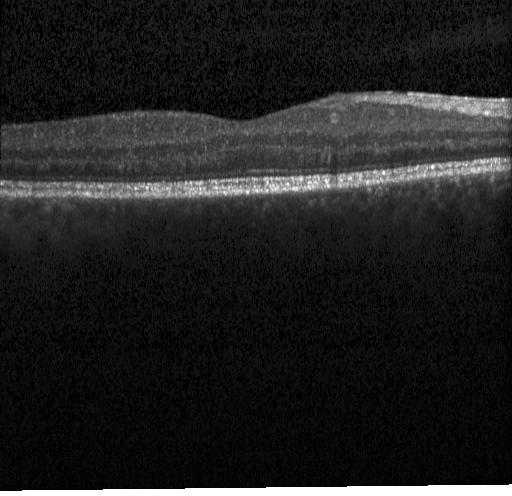
OCT B-scan
OCT finding: no choroidal neovascularization, no diabetic macular edema, and no drusen.